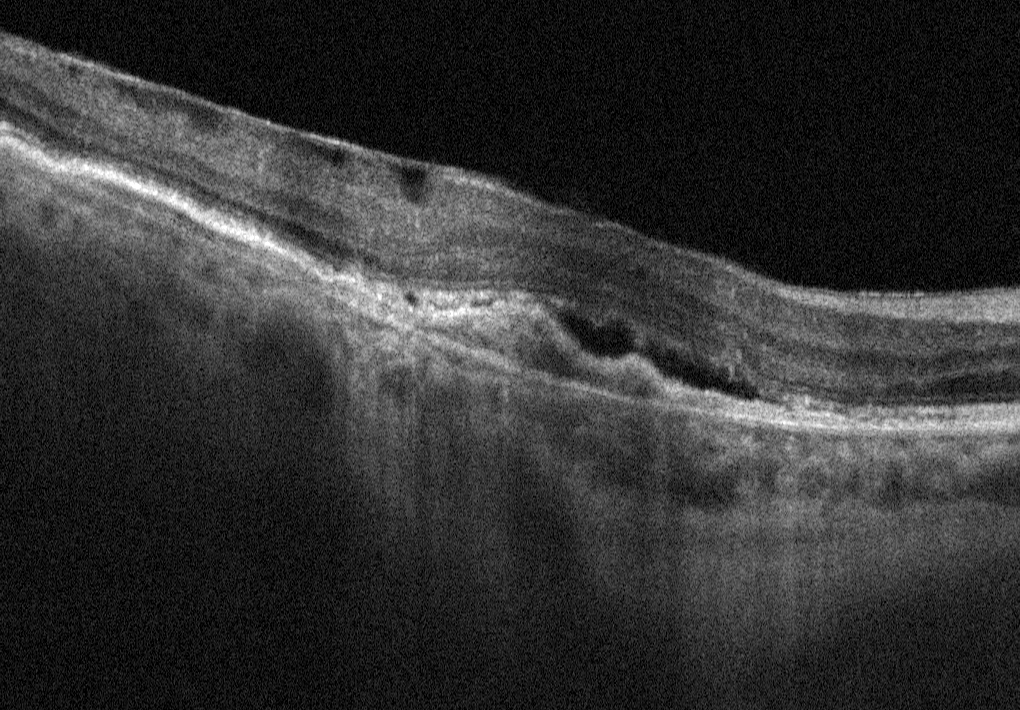 Optical coherence tomography B-scan, through the macula
This B-scan demonstrates AMD.